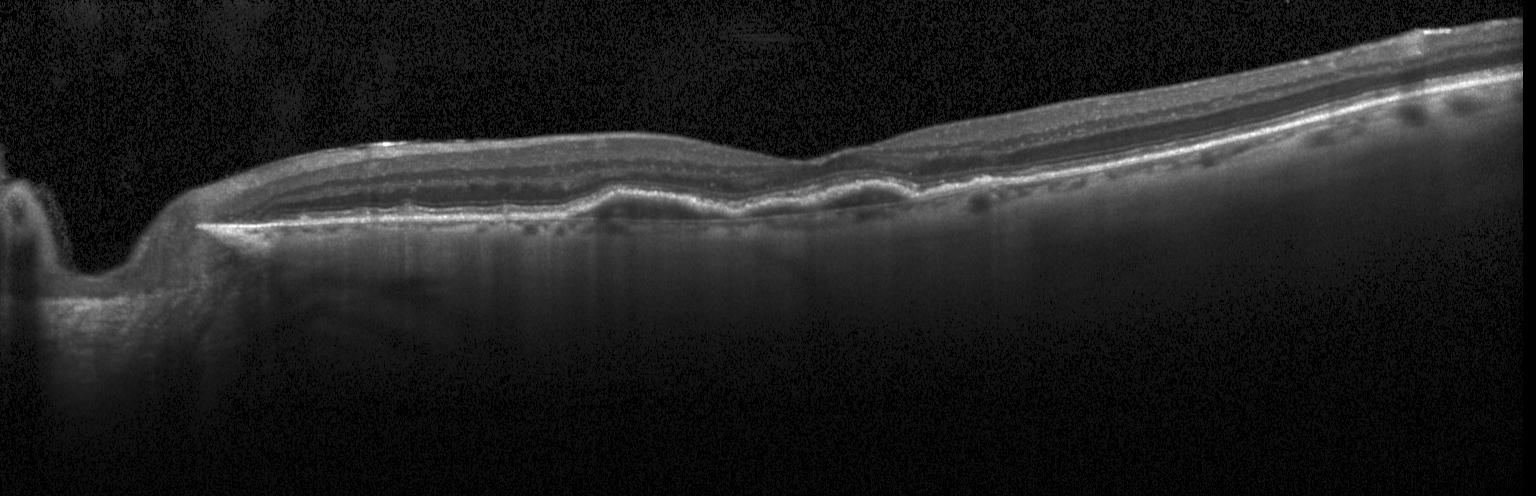
Instrument: Heidelberg Spectralis; spectral-domain OCT; optical coherence tomography scan.
The scan shows a choroidal neovascular membrane.